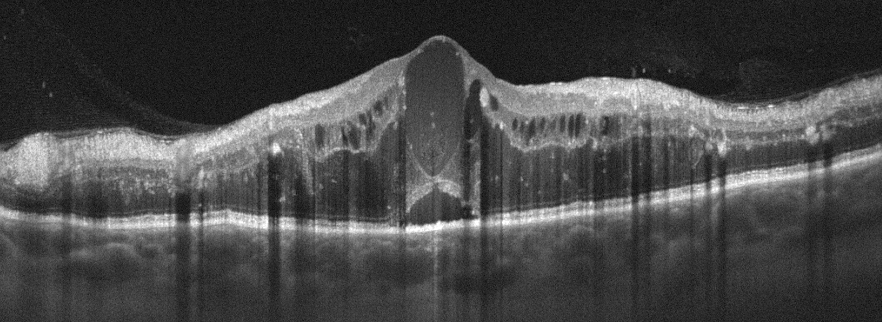

Macular scan. Retinal OCT cross-section. Instrument: Optovue Avanti RTVue XR.
Assessment: retinal vein occlusion (RVO).